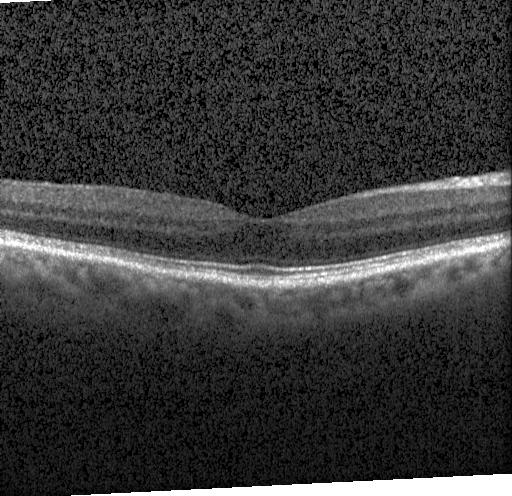
Finding: no choroidal neovascularization, no diabetic macular edema, and no drusen.